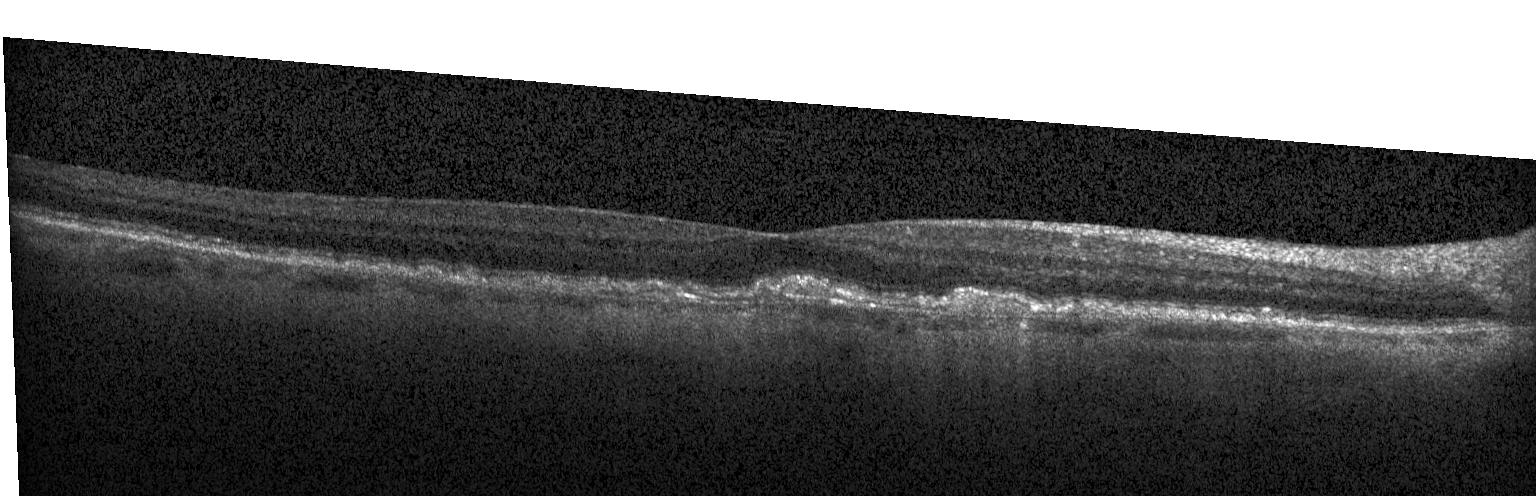

Dx: choroidal neovascularization.